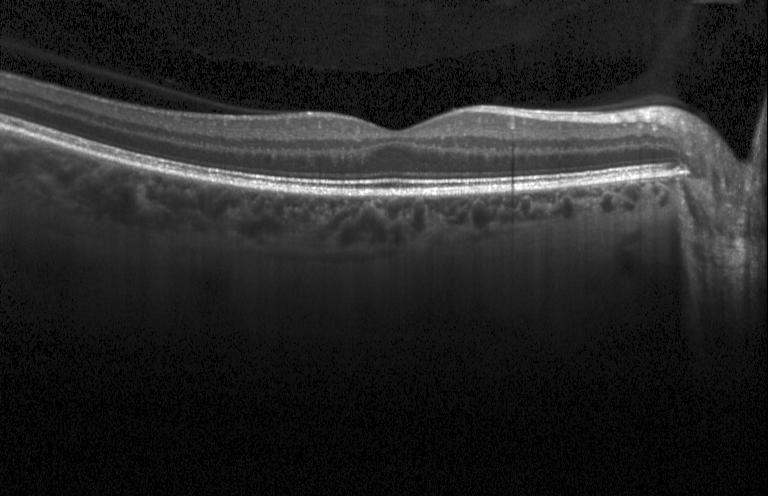
Retinal OCT cross-section · spectral-domain OCT — Impression: no choroidal neovascularization, no diabetic macular edema, and no drusen.